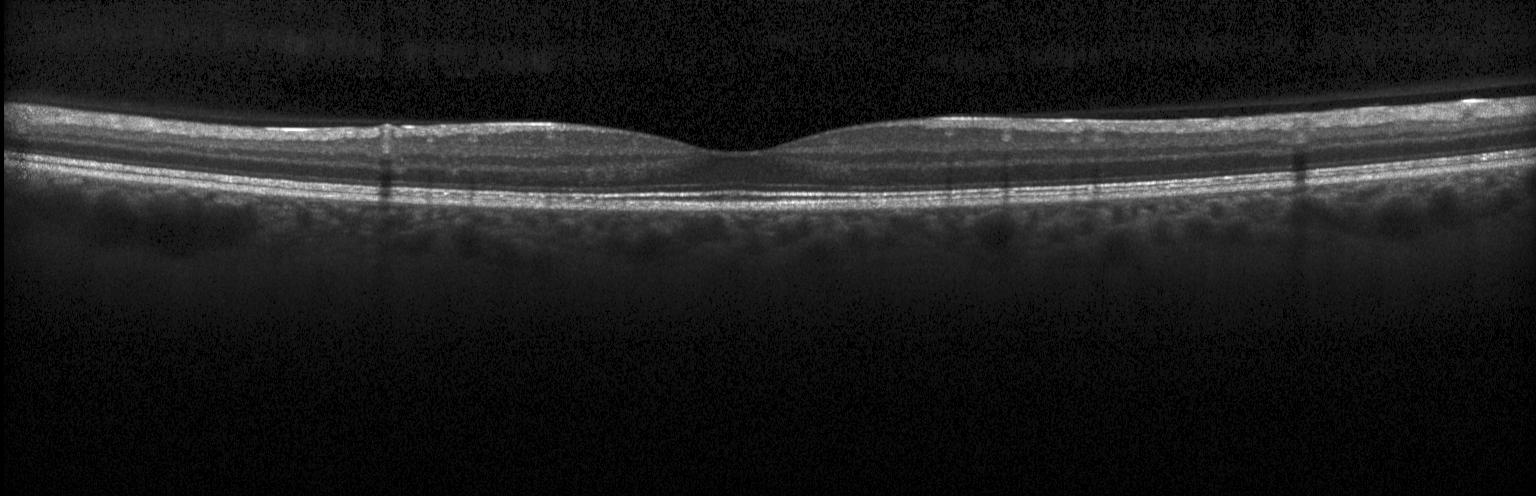 Centered on the fovea; Heidelberg Spectralis; retinal OCT cross-section; spectral-domain optical coherence tomography.
The scan shows no choroidal neovascularization, no diabetic macular edema, and no drusen.